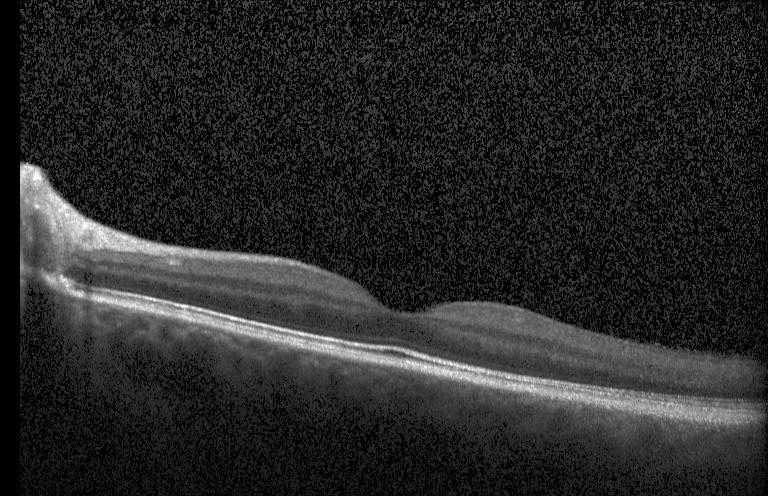
Diagnosis: no choroidal neovascularization, no diabetic macular edema, and no drusen.